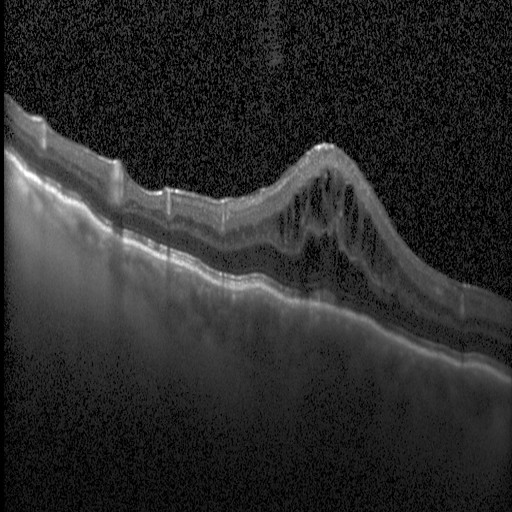 SD-OCT. Retinal OCT B-scan. Instrument: Heidelberg Spectralis.
Diabetic macular edema.